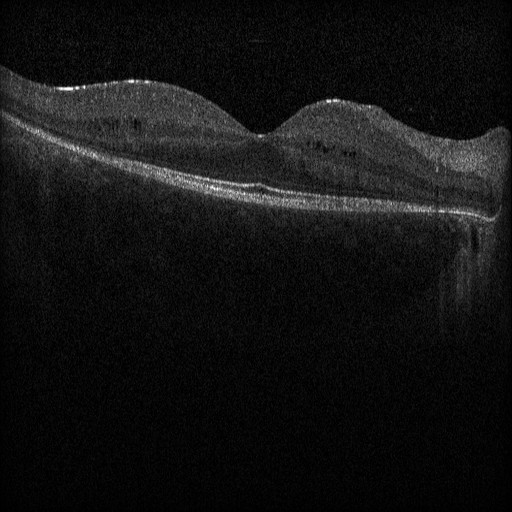
Finding: diabetic macular edema (DME).